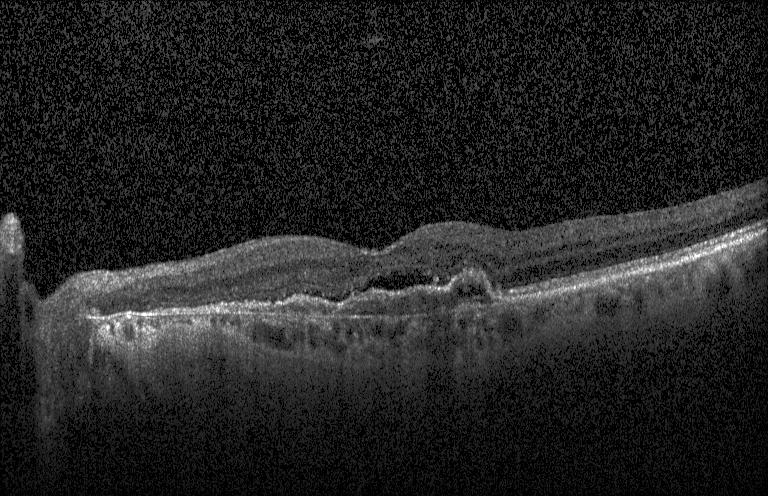
Retinal OCT B-scan.
This B-scan demonstrates choroidal neovascularization.